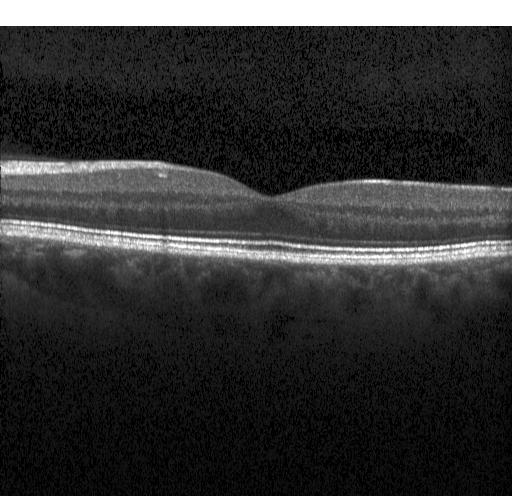
Optical coherence tomography scan. Impression: neither choroidal neovascularization, diabetic macular edema, nor drusen.